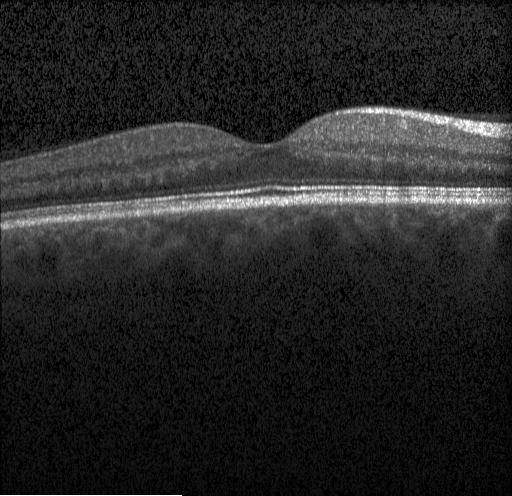

No choroidal neovascularization, diabetic macular edema, or drusen.